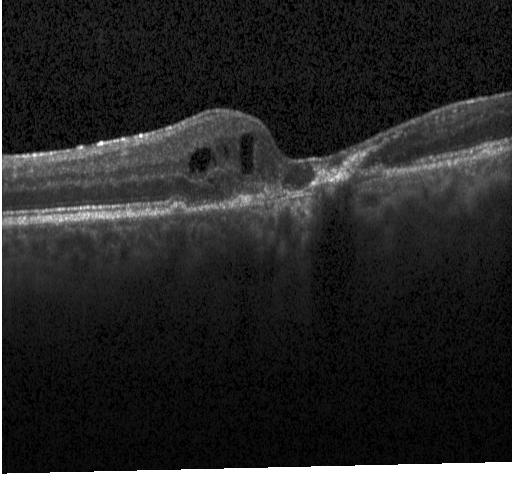
SD-OCT; OCT B-scan; macular scan; acquired on a Heidelberg Spectralis — This B-scan demonstrates choroidal neovascularization (CNV).